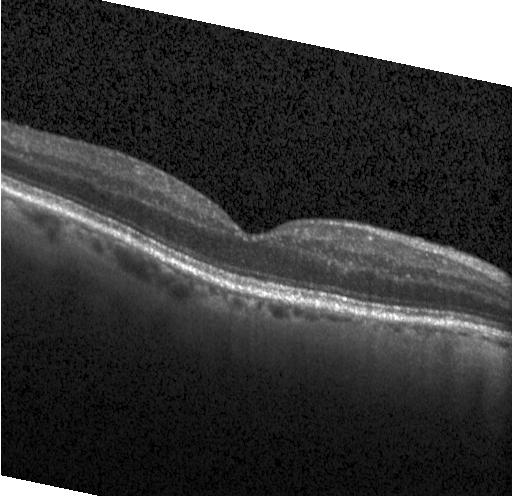
Optical coherence tomography B-scan
No choroidal neovascularization, diabetic macular edema, or drusen.